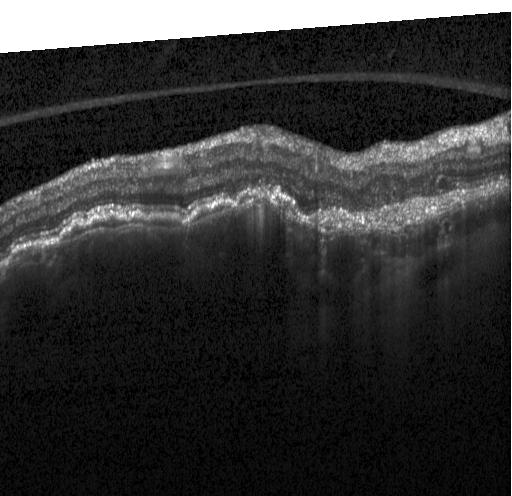 Heidelberg Spectralis. Optical coherence tomography B-scan. Through the macula. SD-OCT
Diagnosis: a choroidal neovascular membrane.